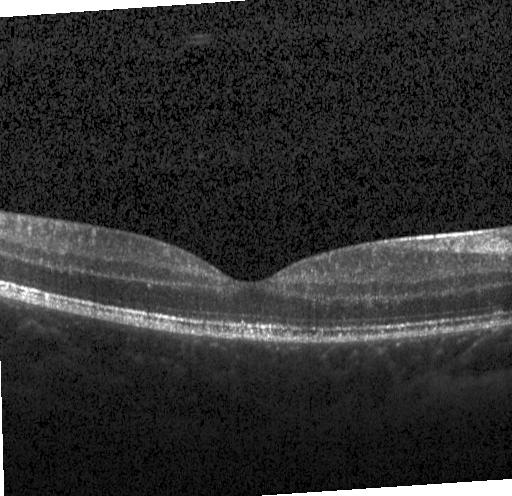
This B-scan demonstrates no evidence of CNV, DME, or drusen.